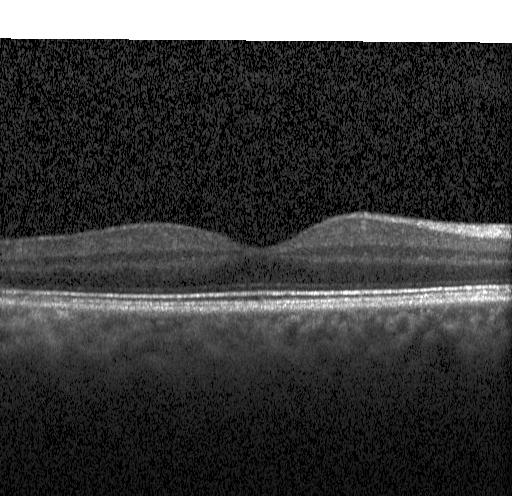 Finding: no choroidal neovascularization, diabetic macular edema, or drusen.